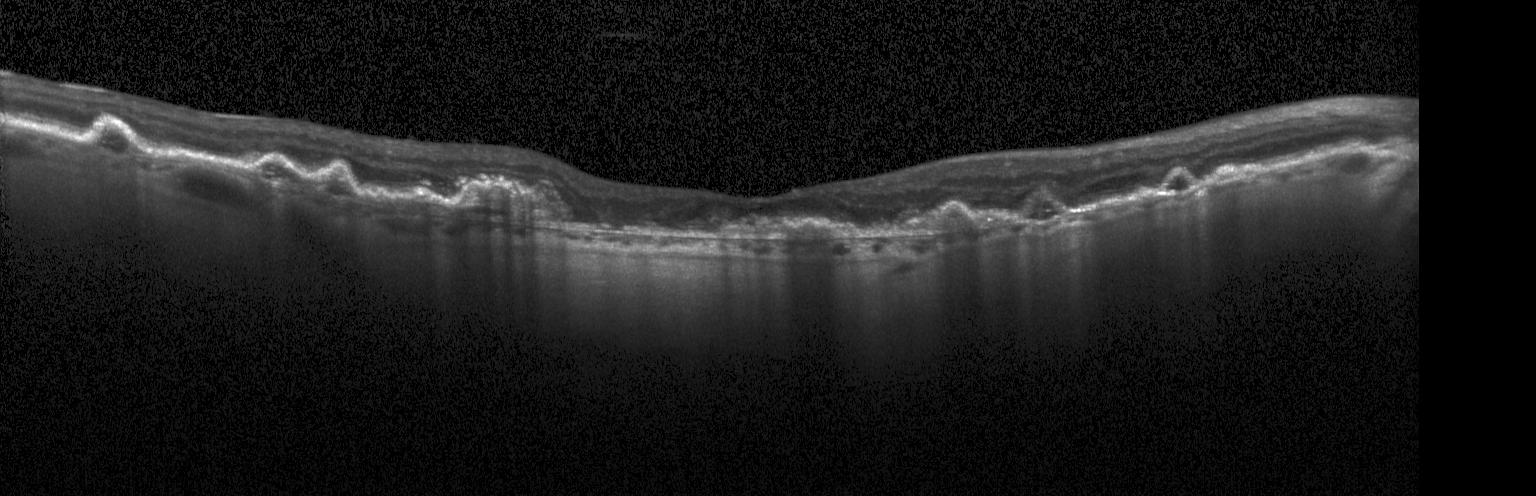

OCT B-scan. Horizontal scan through the fovea — Impression: CNV.